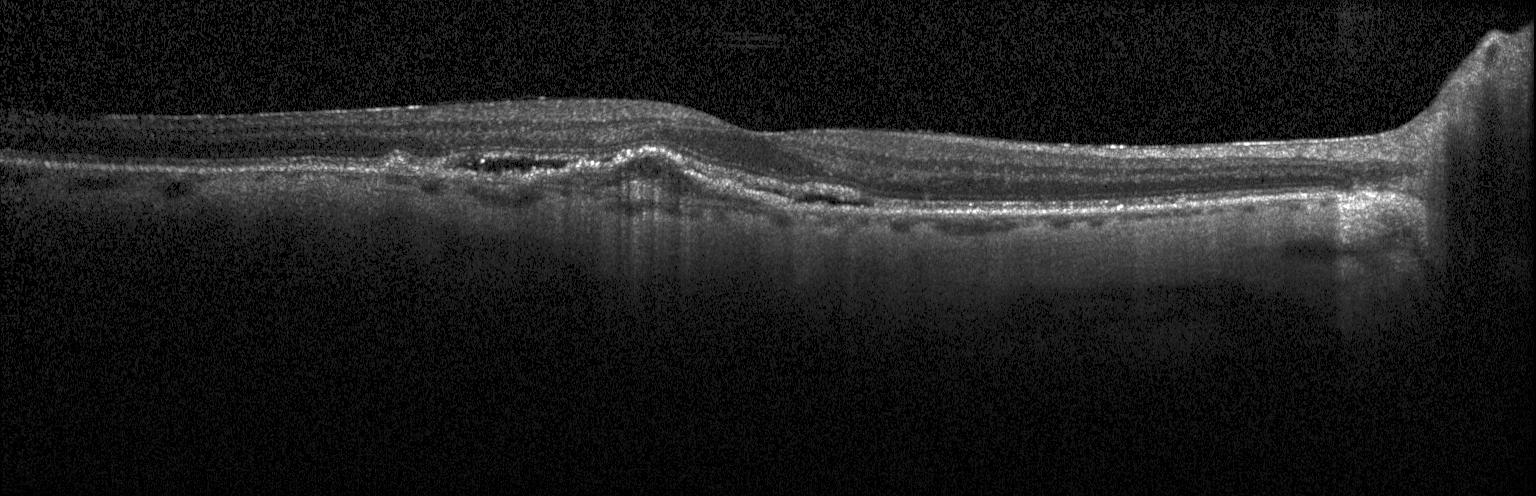 Macular OCT: CNV.